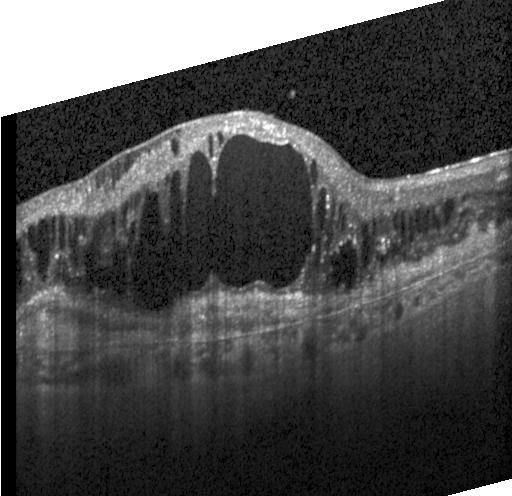
Optical coherence tomography B-scan
Assessment: a choroidal neovascular membrane.